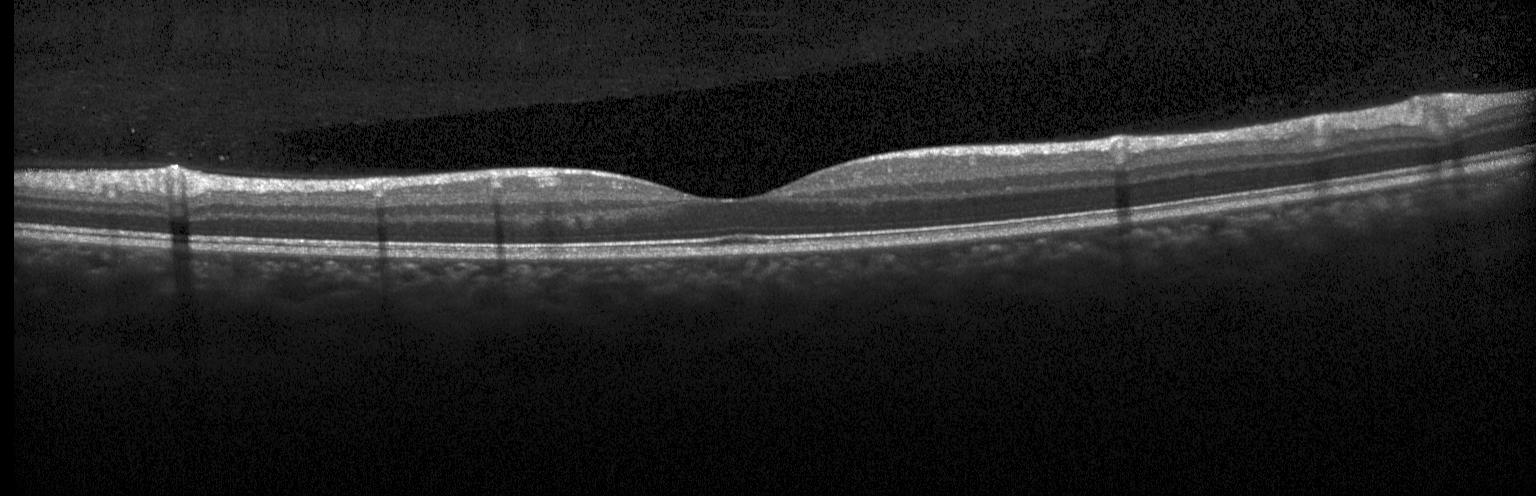

Spectral-domain OCT B-scan: neither choroidal neovascularization, diabetic macular edema, nor drusen.